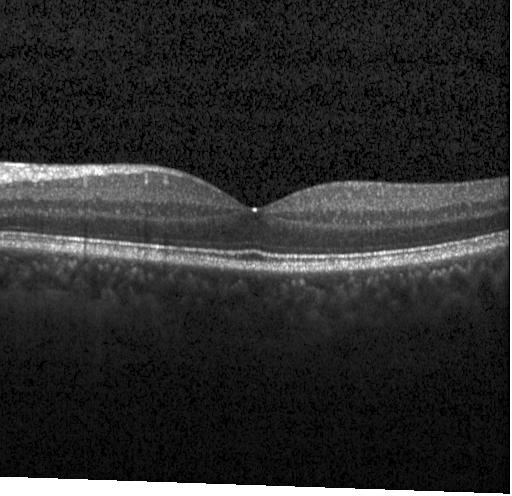 Impression: no CNV, DME, or drusen.